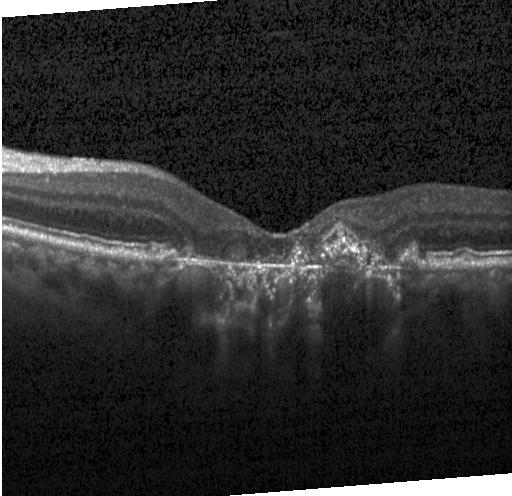 Horizontal scan through the fovea · optical coherence tomography scan — Impression: a choroidal neovascular membrane.